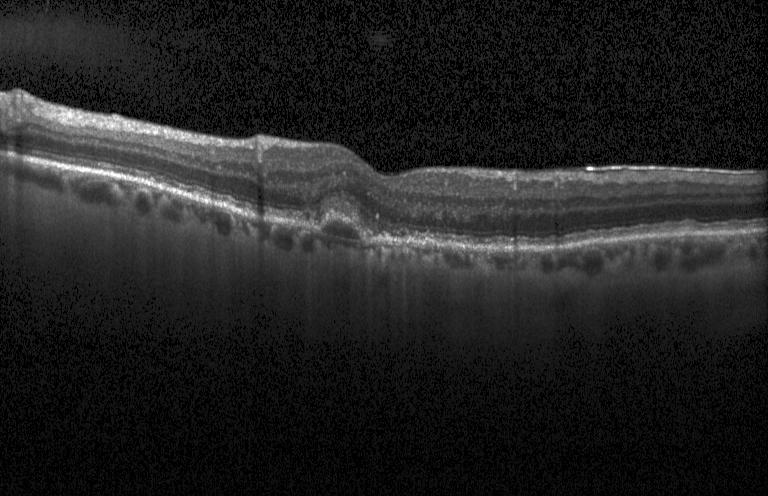 Retinal OCT B-scan, spectral-domain OCT
Macular OCT: a choroidal neovascular membrane.